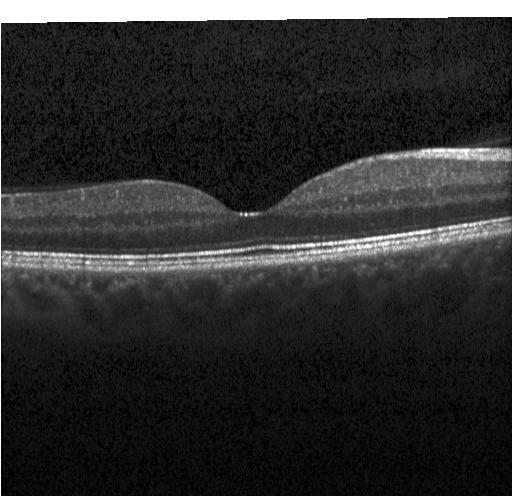 Spectral-domain OCT B-scan: no CNV, DME, or drusen.